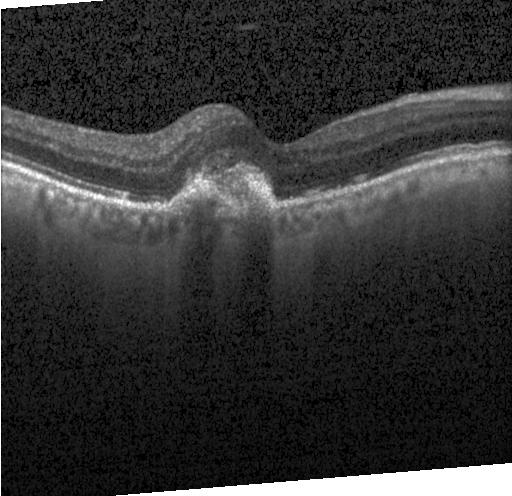 OCT finding: choroidal neovascularization (CNV).